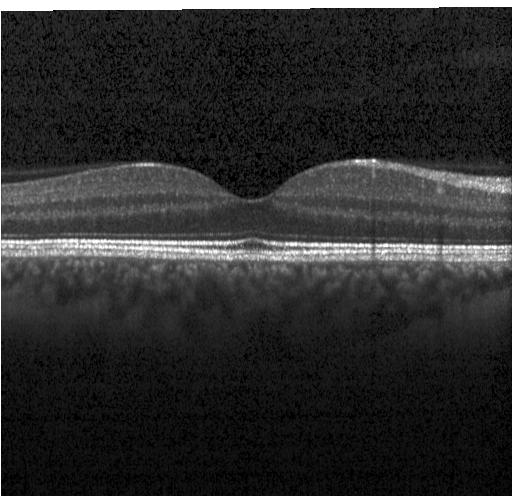 Retinal OCT B-scan.
Dx: no evidence of choroidal neovascularization, diabetic macular edema, or drusen.